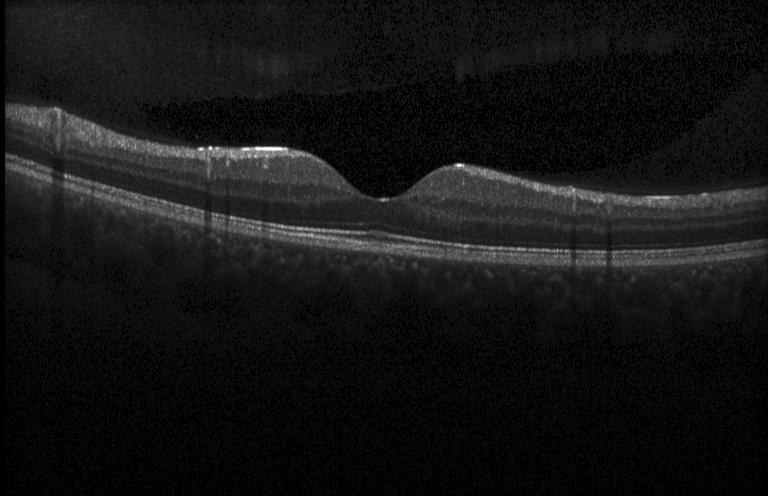 Heidelberg Spectralis OCT system; SD-OCT; OCT line scan
Impression: no CNV, DME, or drusen.